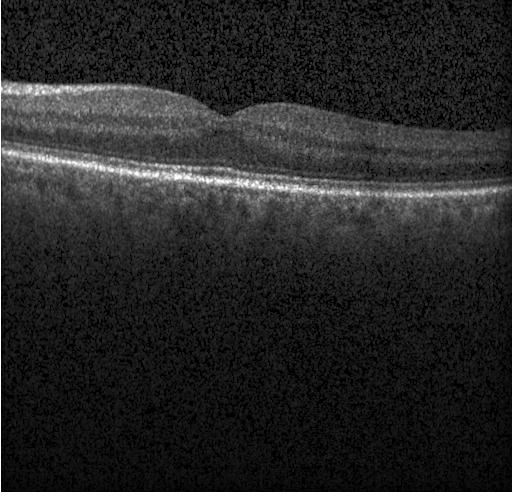
Heidelberg Spectralis. Retinal OCT cross-section. Spectral-domain optical coherence tomography. Fovea-centered
Diagnosis: no CNV, DME, or drusen.